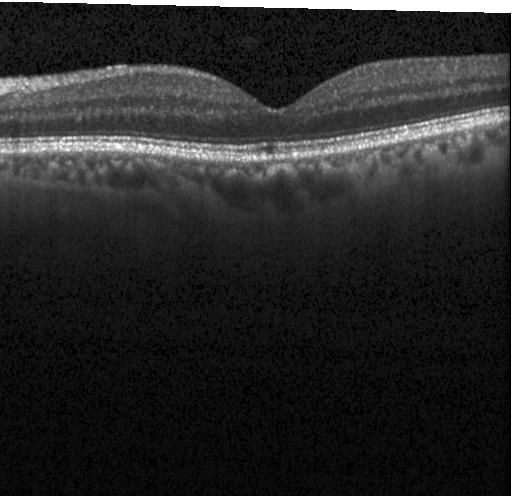

Macular OCT: neither choroidal neovascularization, diabetic macular edema, nor drusen.